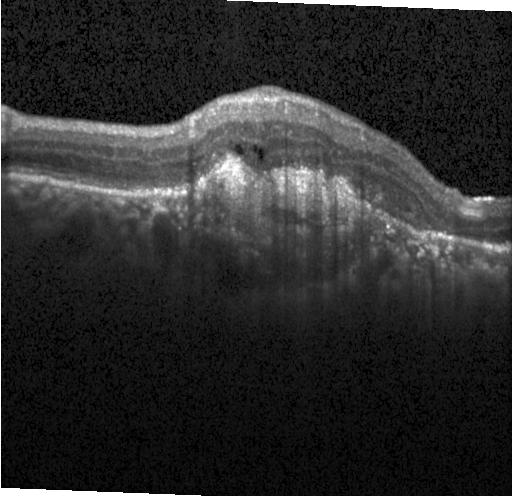

This B-scan demonstrates CNV.